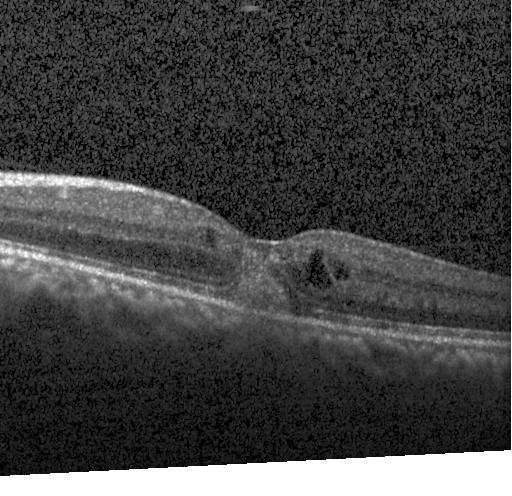 Retinal OCT B-scan.
OCT finding: a choroidal neovascular membrane.